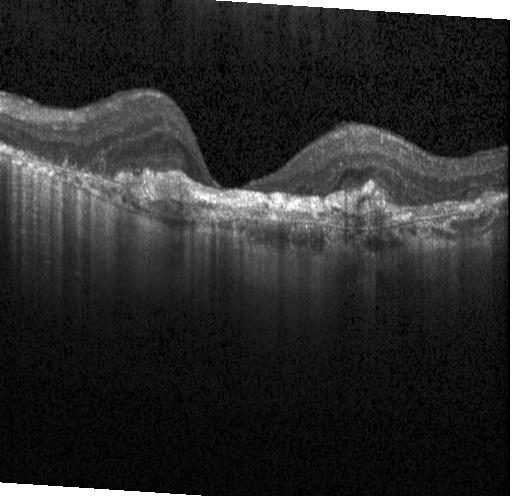
Retinal OCT B-scan, spectral-domain optical coherence tomography.
Dx: a choroidal neovascular membrane.